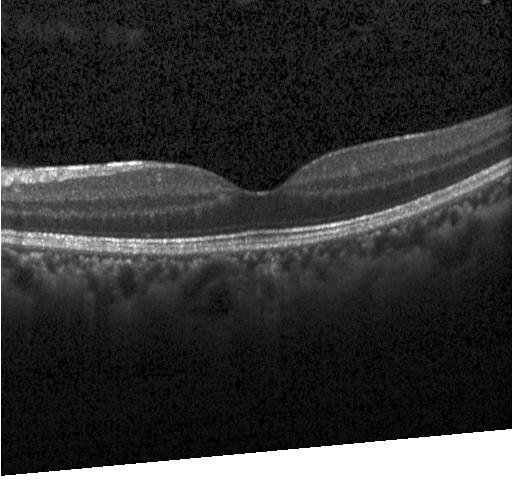 Optical coherence tomography scan. Diagnosis: no CNV, no DME, and no drusen.